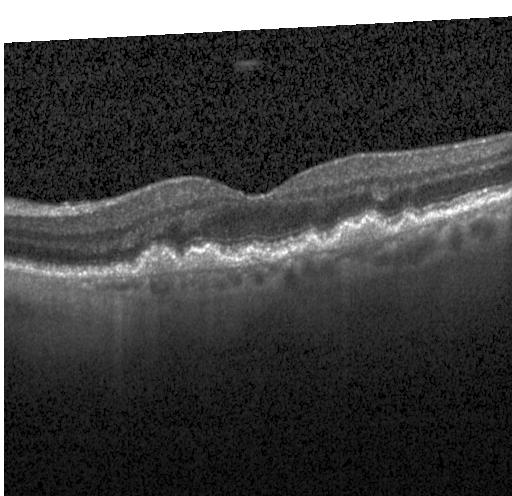 Finding: drusen.